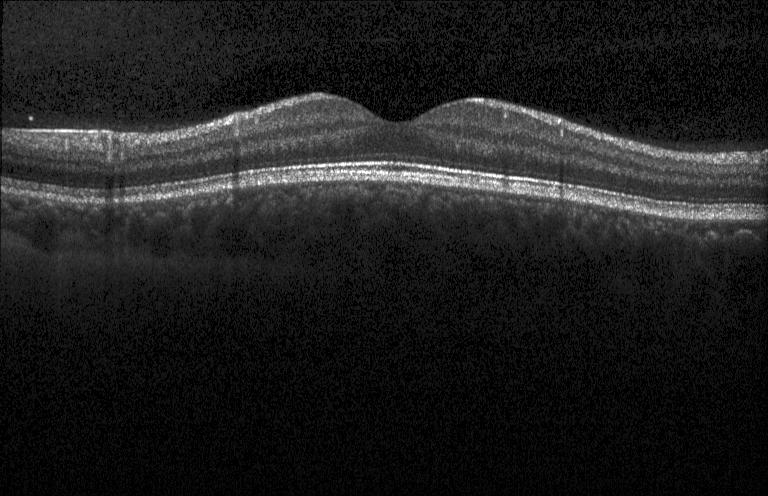
Finding: neither choroidal neovascularization, diabetic macular edema, nor drusen.